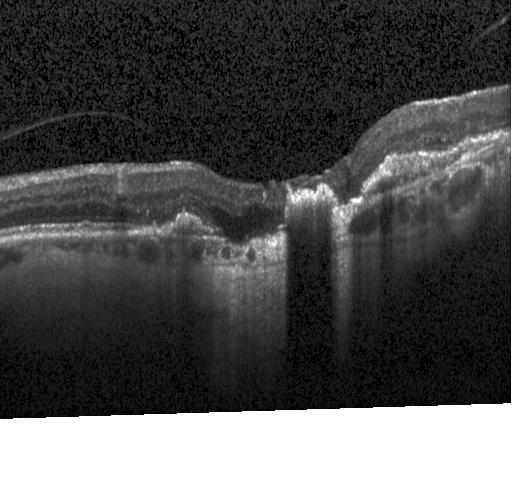

Through the macula. Optical coherence tomography scan.
OCT finding: choroidal neovascularization (CNV).